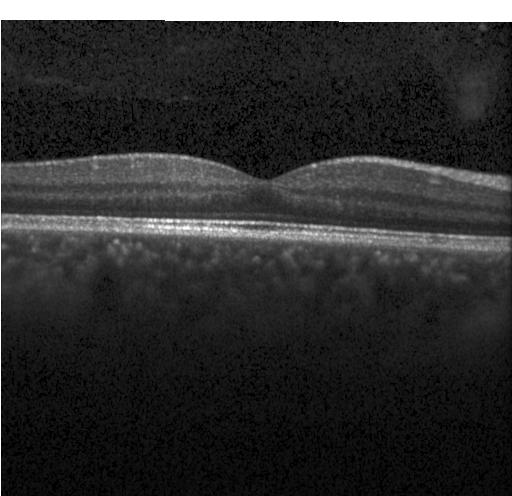

Heidelberg Spectralis OCT system · spectral-domain OCT · horizontal scan through the fovea · optical coherence tomography B-scan.
Impression: no evidence of choroidal neovascularization, diabetic macular edema, or drusen.